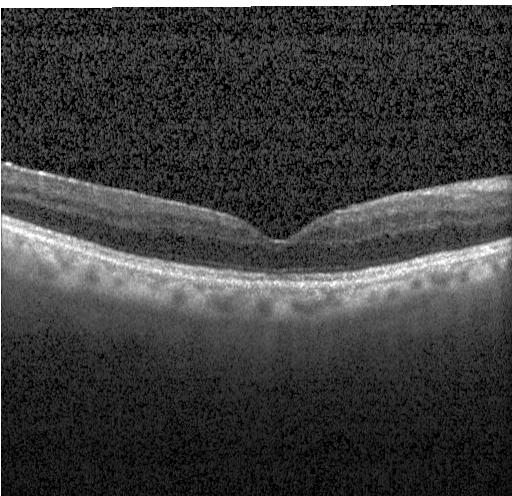
Optical coherence tomography B-scan — OCT finding: neither CNV, DME, nor drusen.